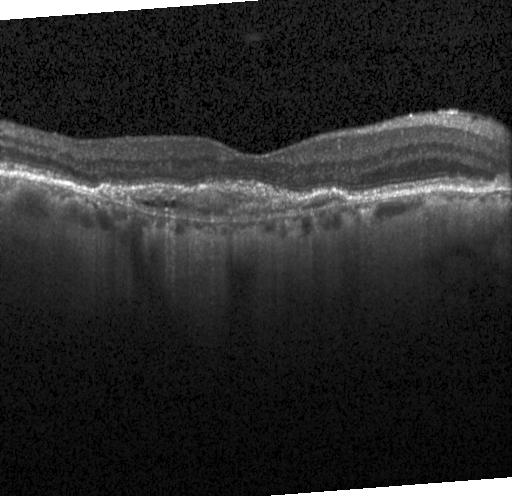
OCT line scan · acquired on a Heidelberg Spectralis · through the macula · spectral-domain OCT
OCT finding: choroidal neovascularization (CNV).